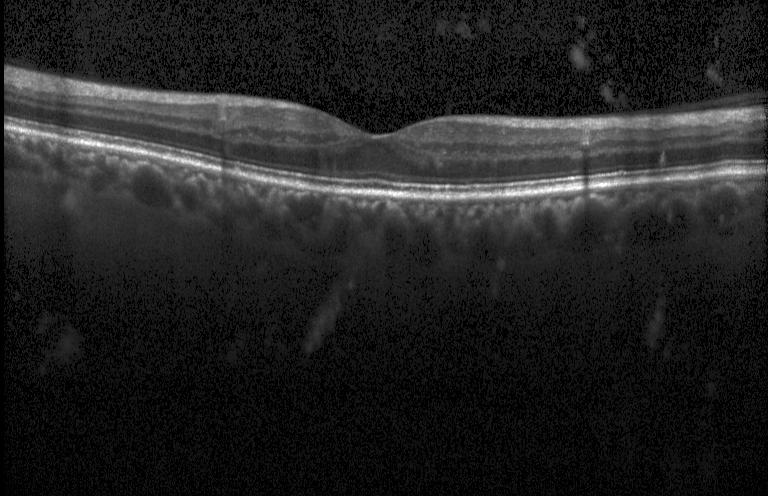 Finding: no choroidal neovascularization, no diabetic macular edema, and no drusen.